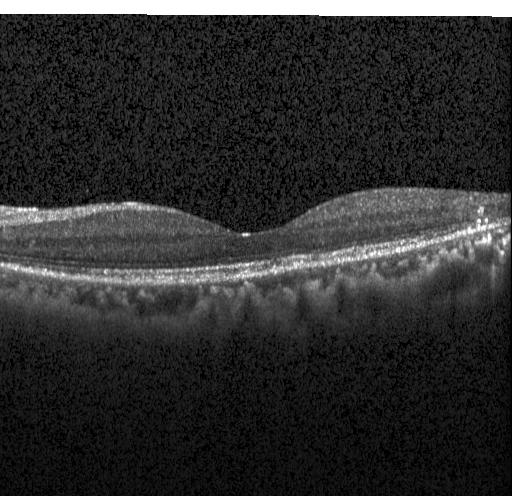 OCT line scan. No choroidal neovascularization, no diabetic macular edema, and no drusen.